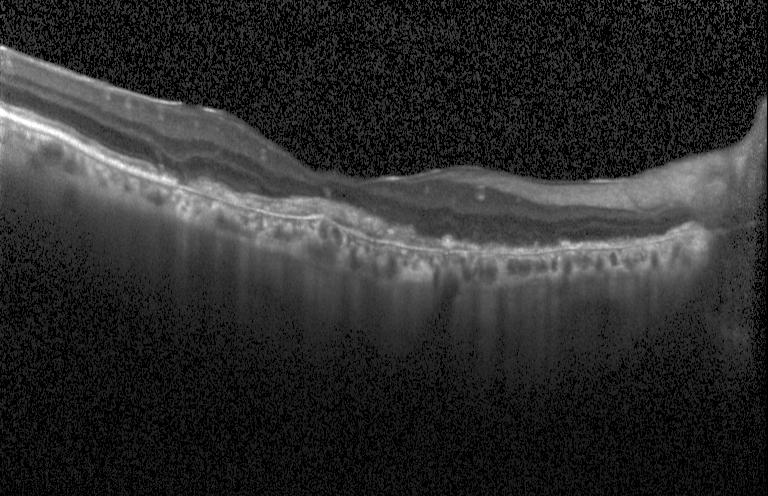 Retinal OCT B-scan · horizontal scan through the fovea · Heidelberg Spectralis OCT system · spectral-domain optical coherence tomography — Impression: choroidal neovascularization.